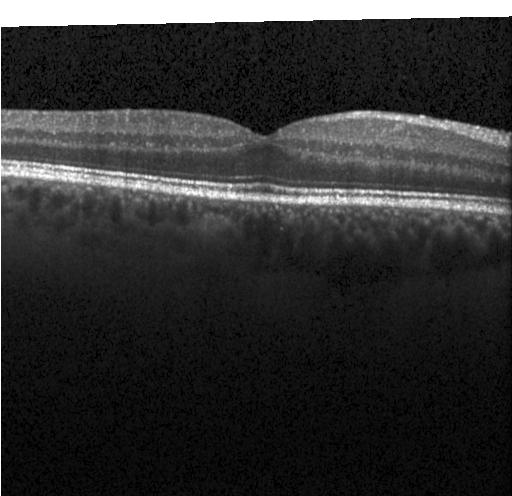
Heidelberg Spectralis · optical coherence tomography B-scan · horizontal scan through the fovea · spectral-domain OCT. Diagnosis: no choroidal neovascularization, diabetic macular edema, or drusen.